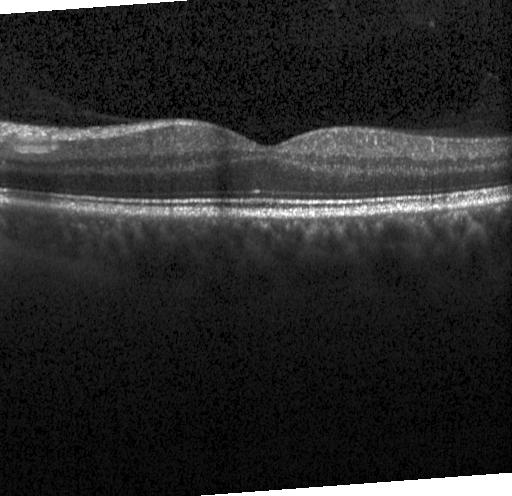
Impression: neither choroidal neovascularization, diabetic macular edema, nor drusen.